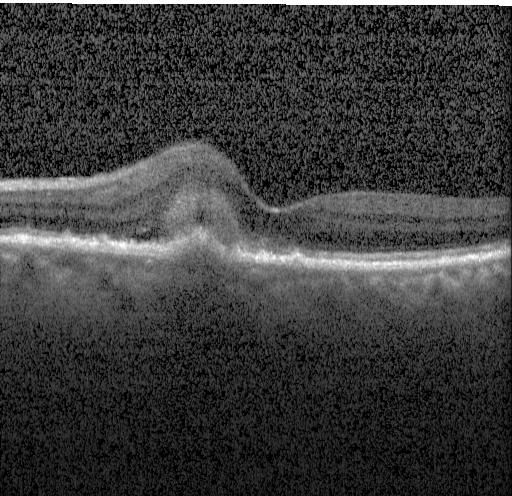 OCT B-scan, acquired on a Heidelberg Spectralis.
CNV.